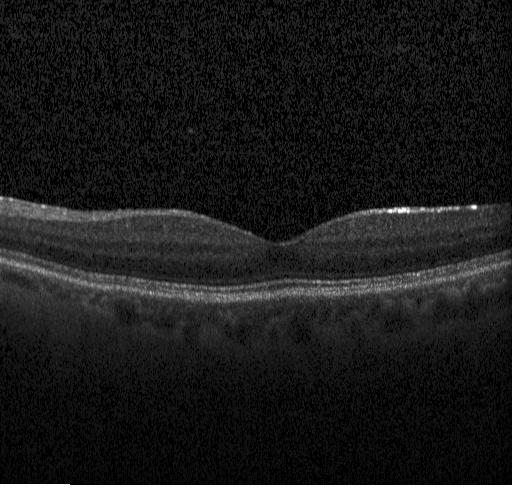 Diagnosis: neither CNV, DME, nor drusen.